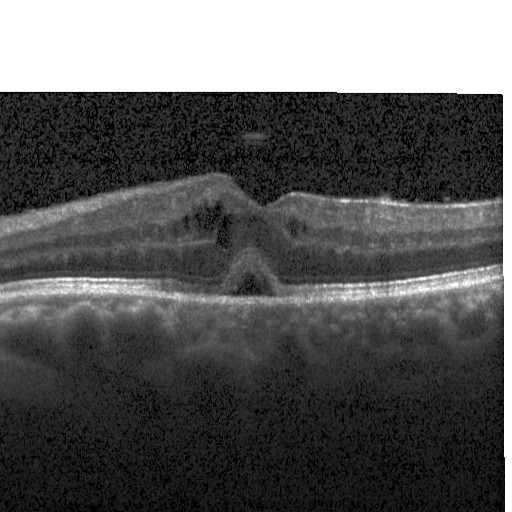 Through the macula. OCT line scan. Instrument: Heidelberg Spectralis. Spectral-domain optical coherence tomography
Assessment: DME.